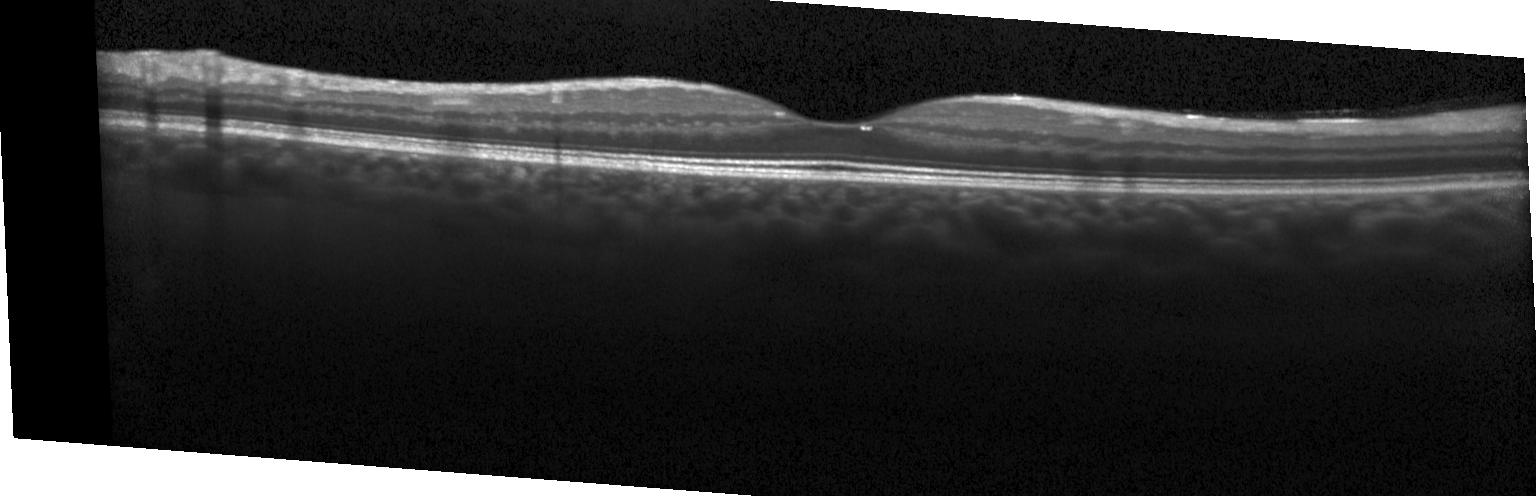 Optical coherence tomography scan; spectral-domain optical coherence tomography.
This B-scan demonstrates neither CNV, DME, nor drusen.